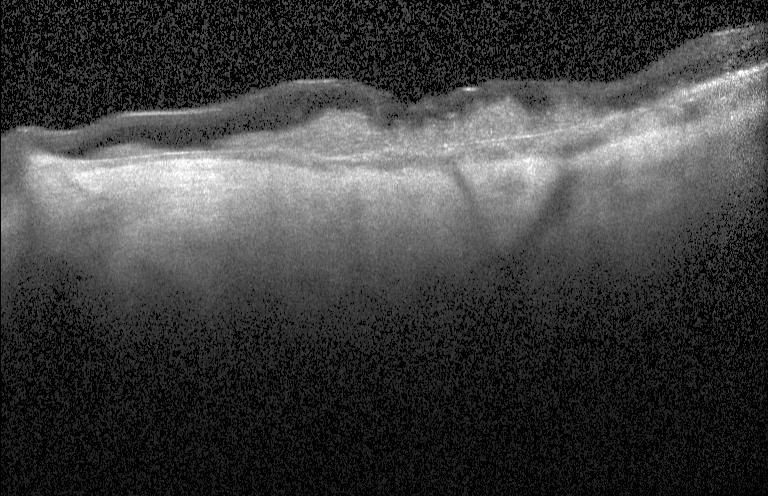

SD-OCT. Optical coherence tomography B-scan. Heidelberg Spectralis OCT system. Macular OCT: choroidal neovascularization.